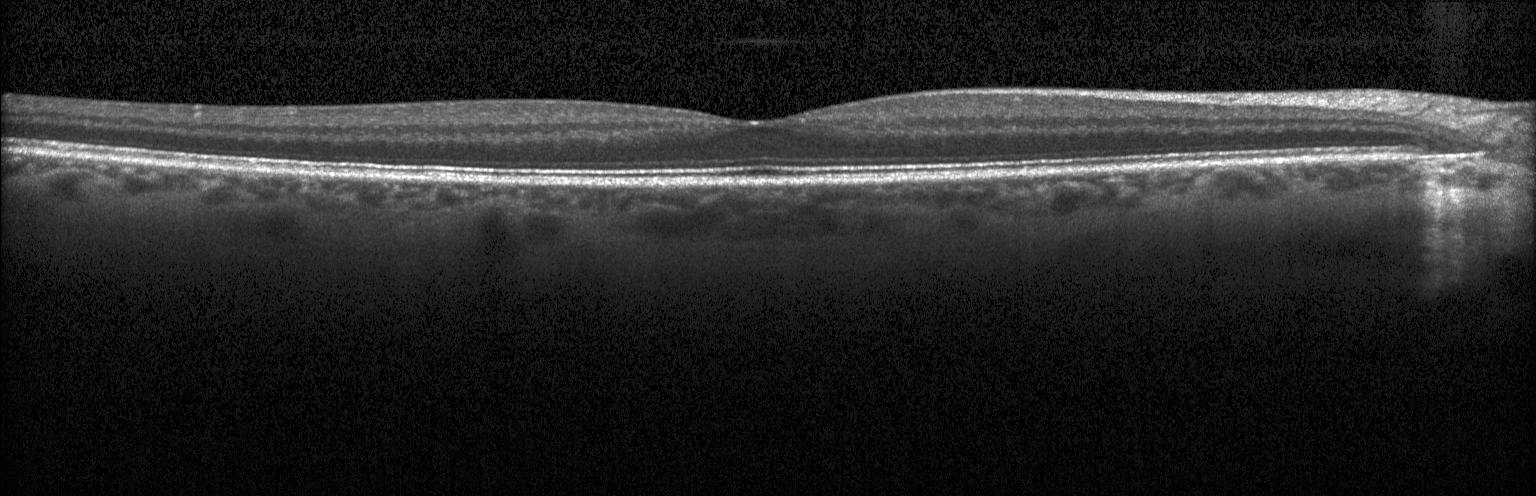
OCT line scan
Diagnosis: no CNV, no DME, and no drusen.